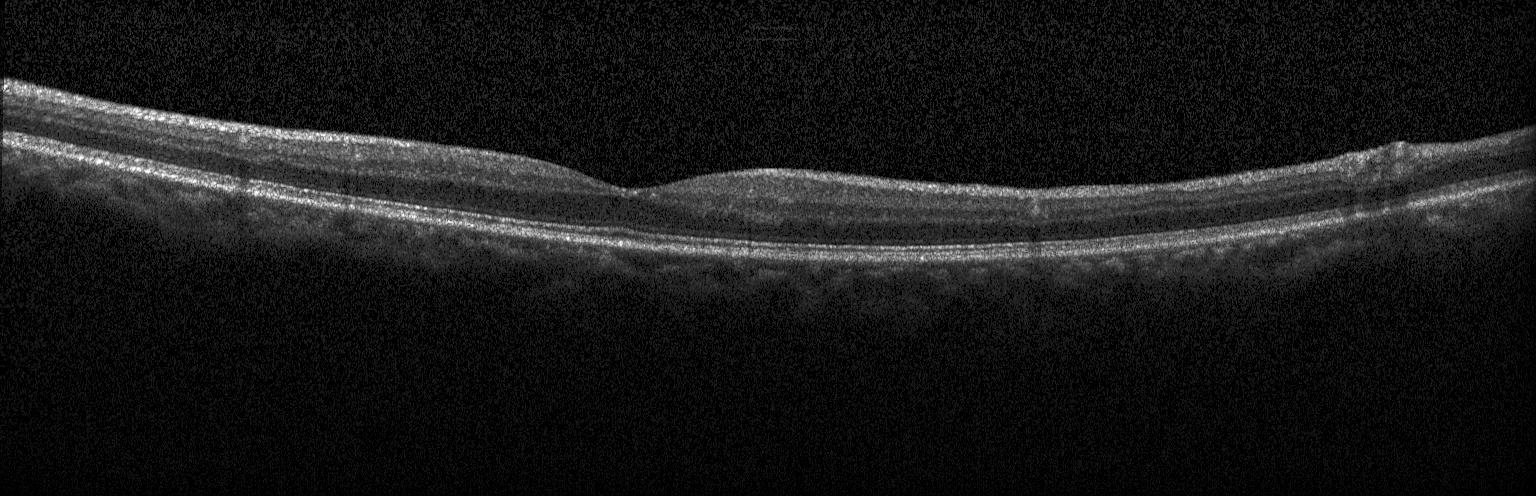

OCT scan showing neither choroidal neovascularization, diabetic macular edema, nor drusen.